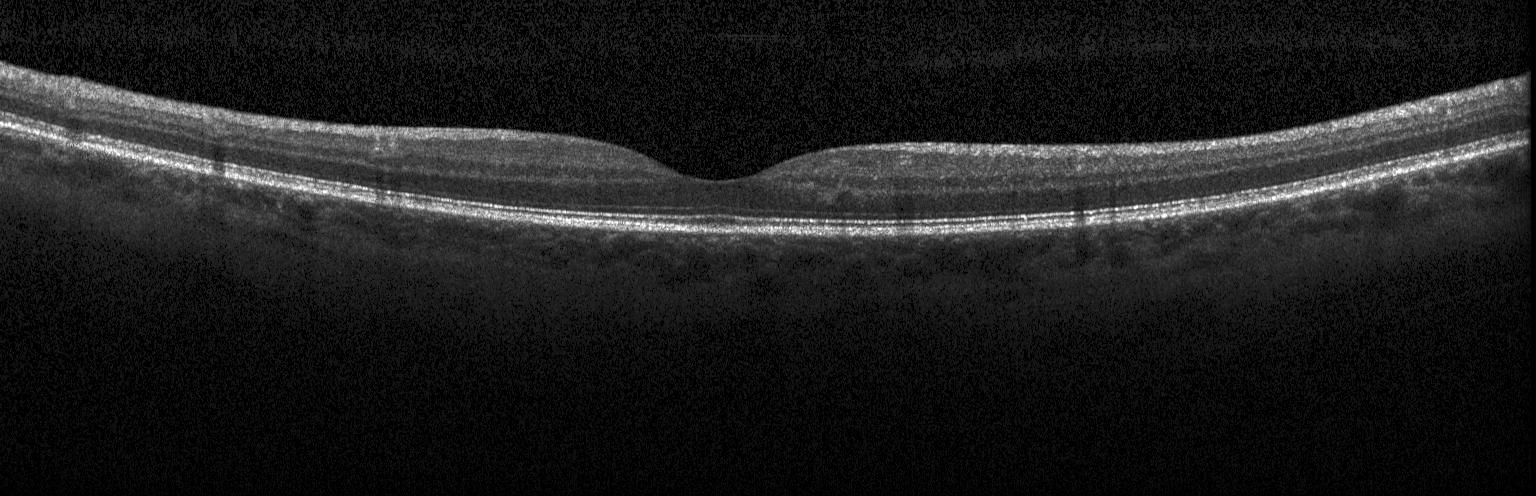
Finding: no CNV, no DME, and no drusen.